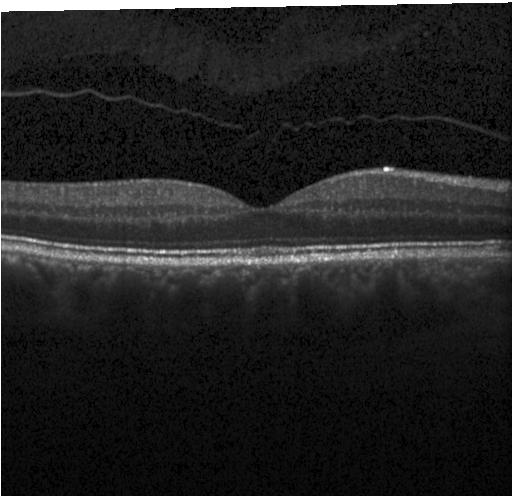

SD-OCT; OCT B-scan; Heidelberg Spectralis
No CNV, DME, or drusen.